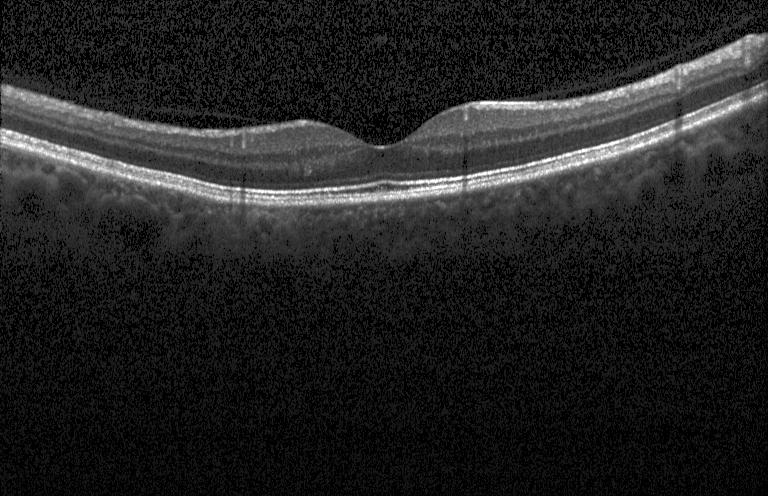

Spectral-domain OCT B-scan: no choroidal neovascularization, no diabetic macular edema, and no drusen.